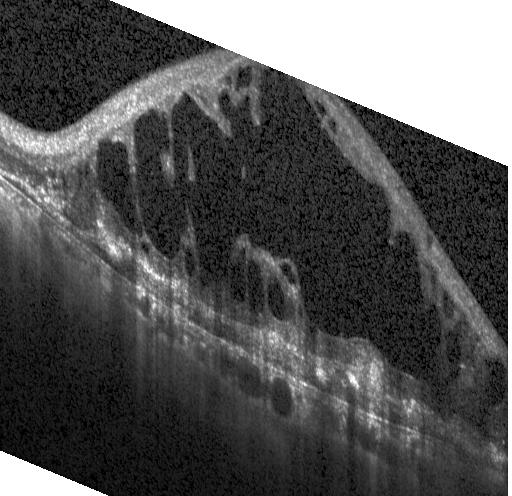 OCT finding: CNV.